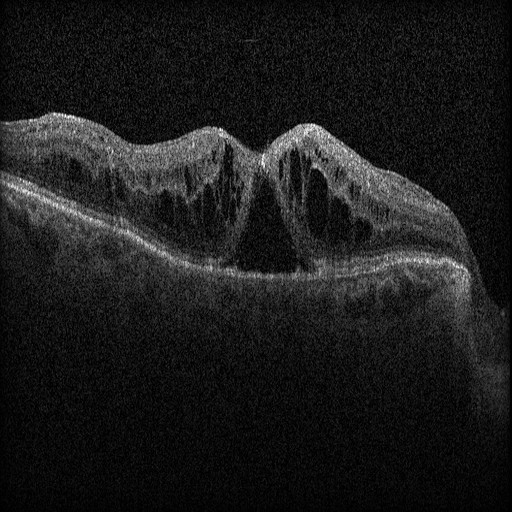
OCT B-scan — Assessment: DME.